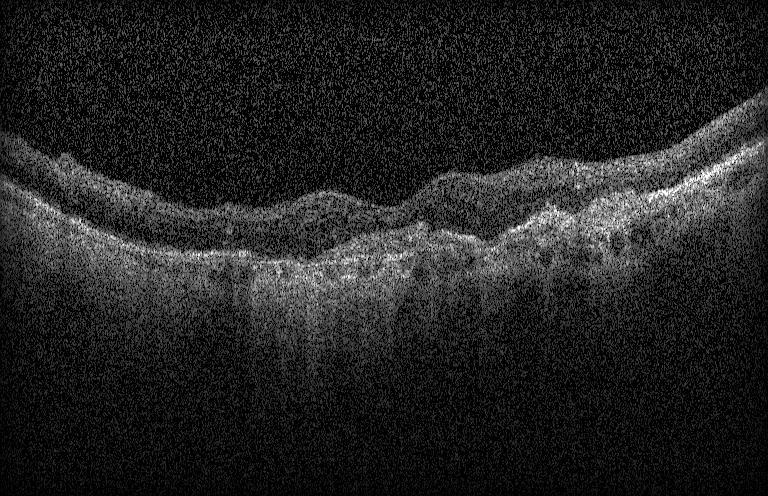 Through the macula, spectral-domain optical coherence tomography, optical coherence tomography scan, instrument: Heidelberg Spectralis
Assessment: choroidal neovascularization.